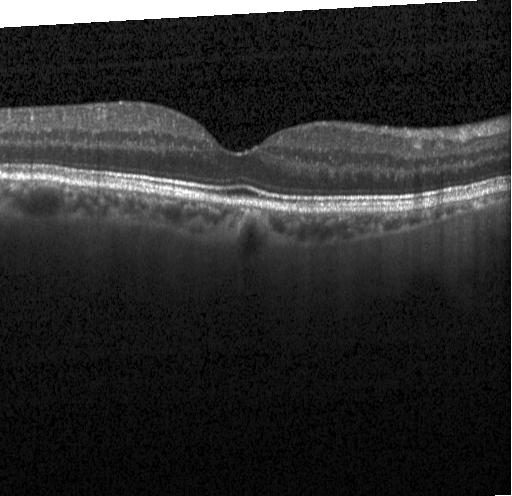
Optical coherence tomography scan. Centered on the fovea. Spectral-domain OCT. Diagnosis: neither choroidal neovascularization, diabetic macular edema, nor drusen.